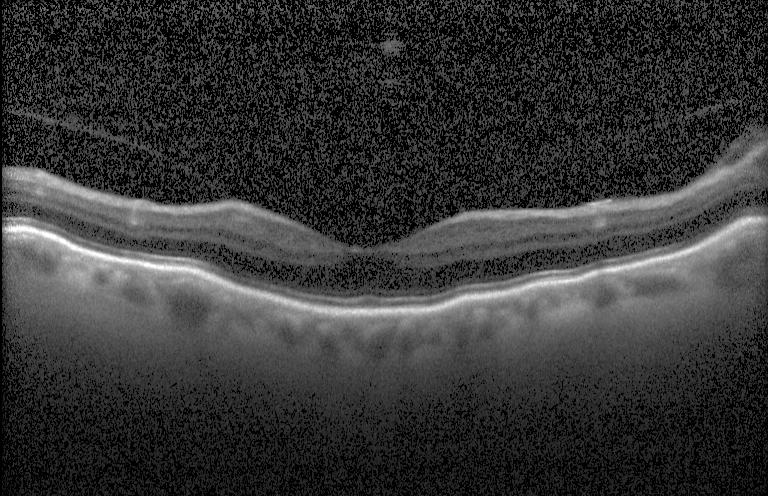

Spectral-domain optical coherence tomography · retinal OCT cross-section · macular scan
Macular OCT: no CNV, DME, or drusen.